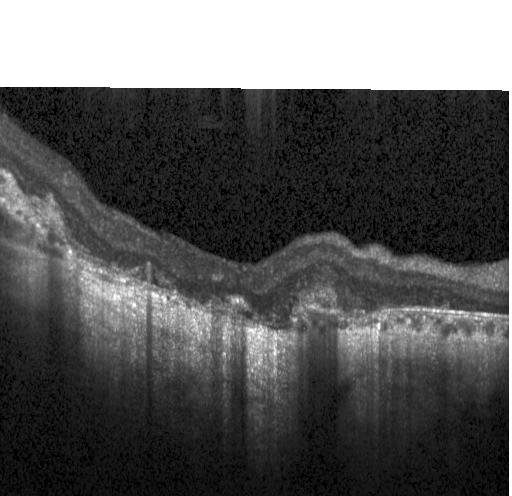 Retinal OCT cross-section.
OCT finding: choroidal neovascularization (CNV).